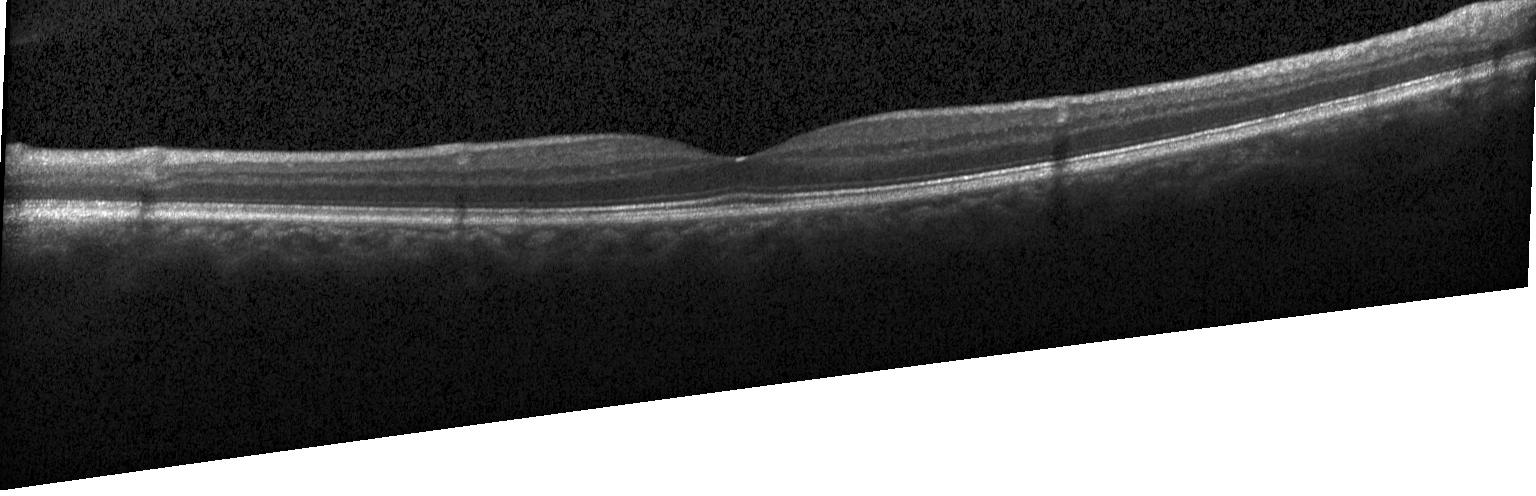
Heidelberg Spectralis; SD-OCT; fovea-centered; optical coherence tomography scan
Impression: neither CNV, DME, nor drusen.